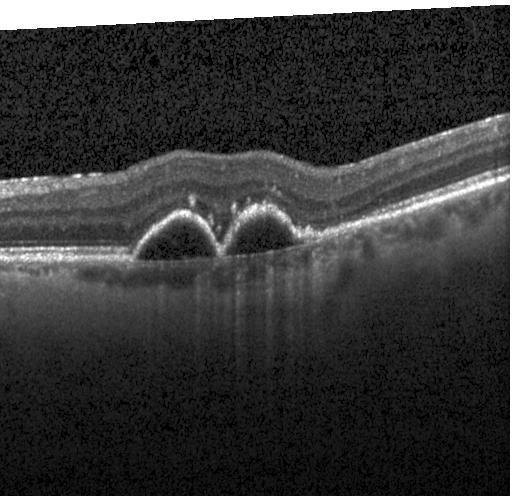

Retinal OCT B-scan. A choroidal neovascular membrane.